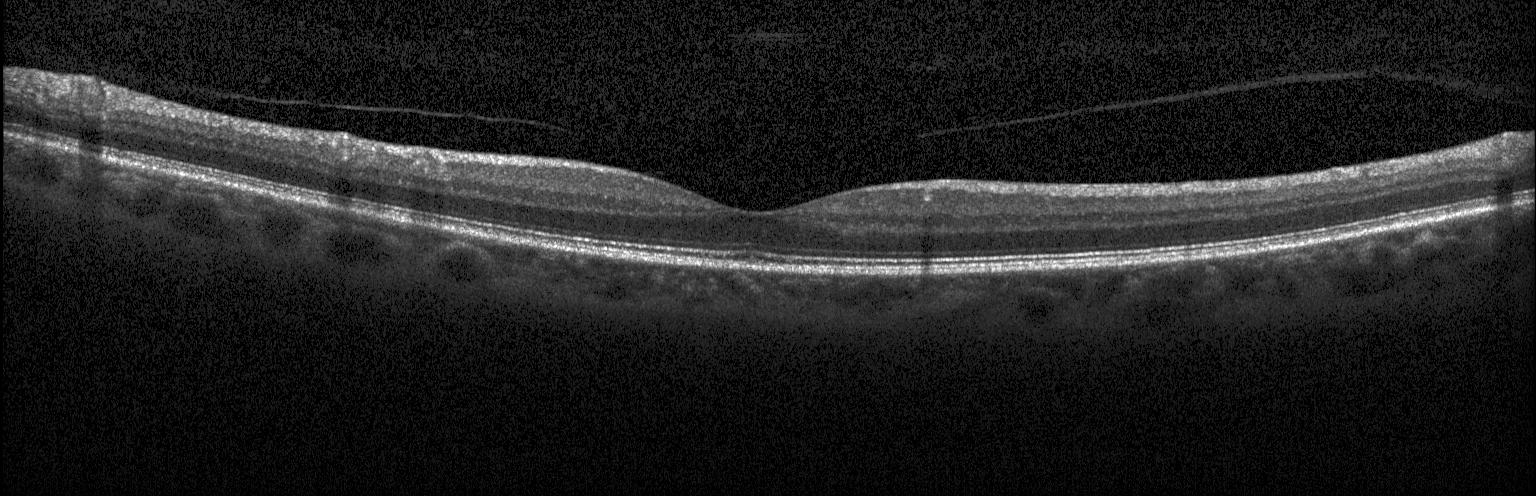 Retinal OCT B-scan · acquired on a Heidelberg Spectralis · spectral-domain optical coherence tomography · macular scan. Macular OCT: no evidence of choroidal neovascularization, diabetic macular edema, or drusen.